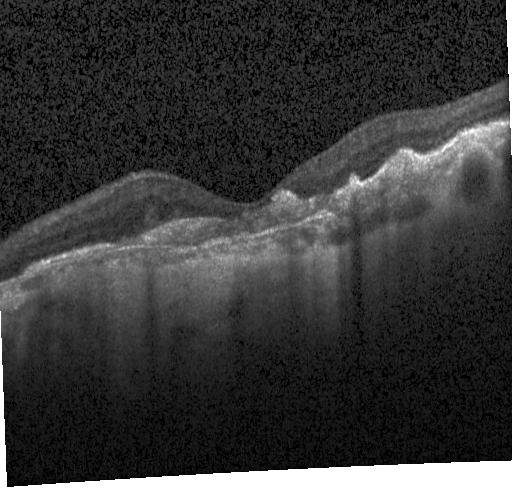
Fovea-centered. Spectral-domain OCT. Optical coherence tomography scan. Assessment: a choroidal neovascular membrane.